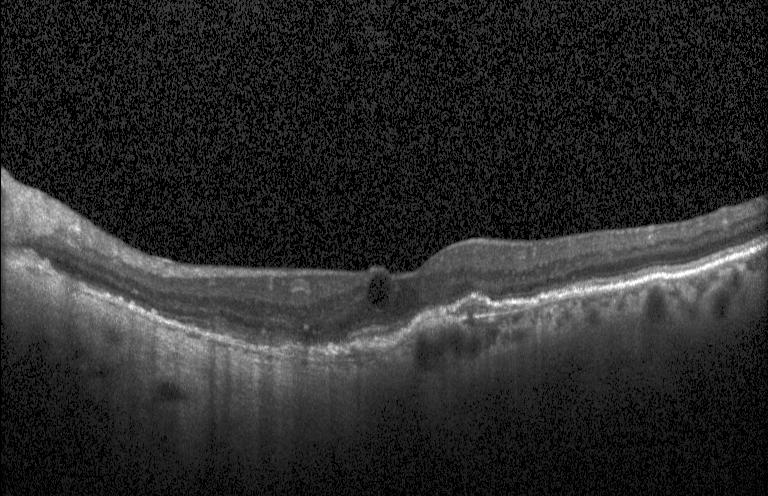
Dx: CNV.